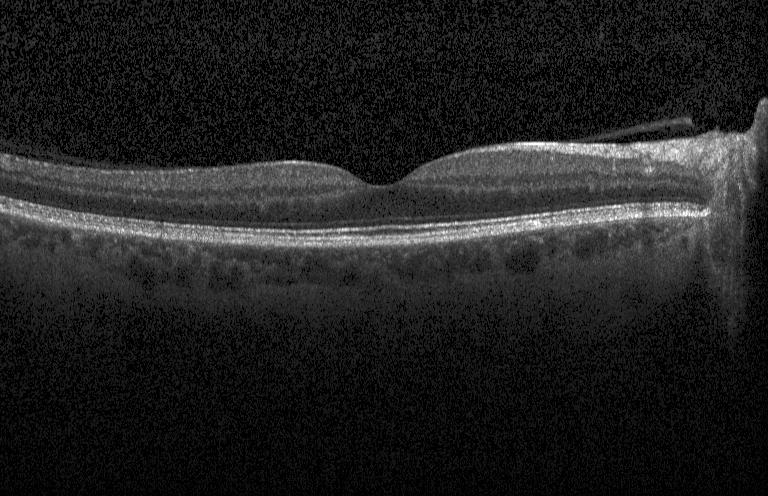
Optical coherence tomography B-scan. Heidelberg Spectralis OCT system. Centered on the fovea
Diagnosis: no evidence of choroidal neovascularization, diabetic macular edema, or drusen.